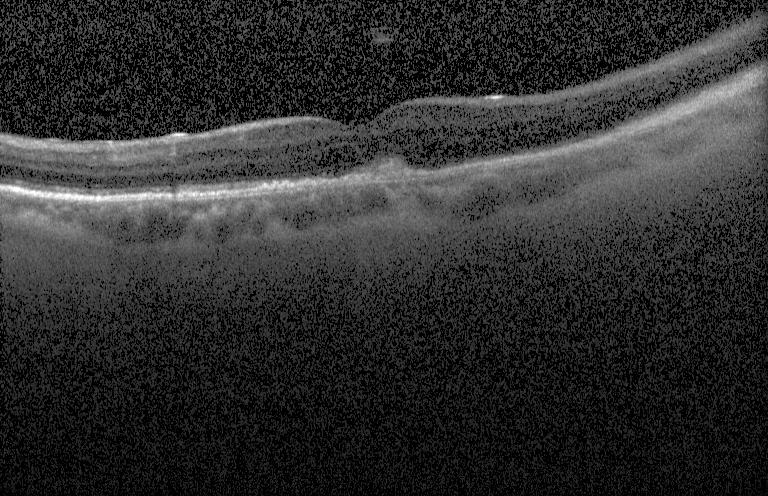 OCT line scan.
Diagnosis: CNV.